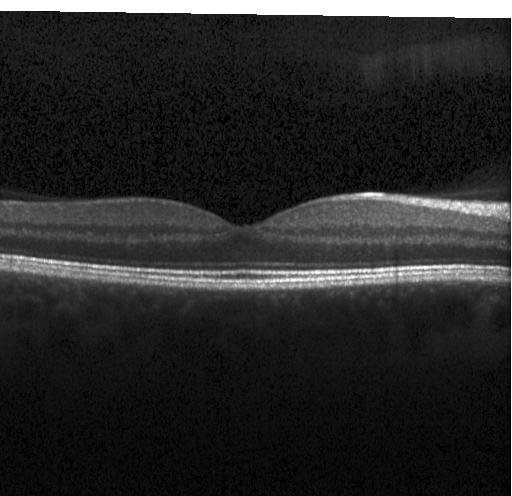 Spectral-domain OCT B-scan: no choroidal neovascularization, no diabetic macular edema, and no drusen.